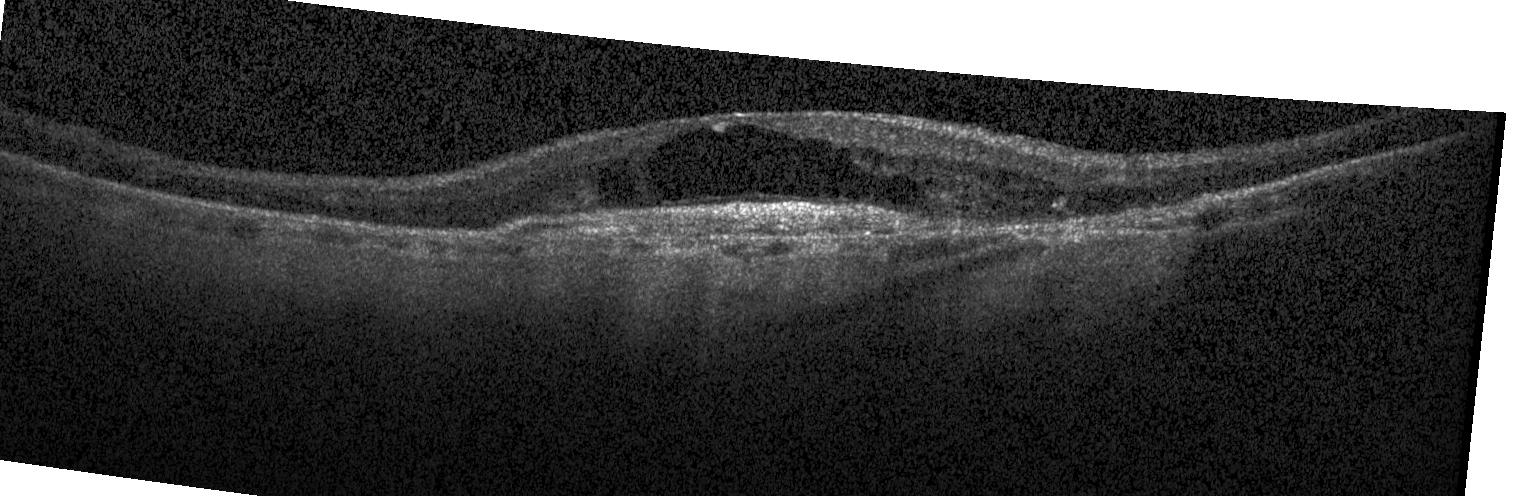
Optical coherence tomography scan, fovea-centered — Macular OCT: CNV.